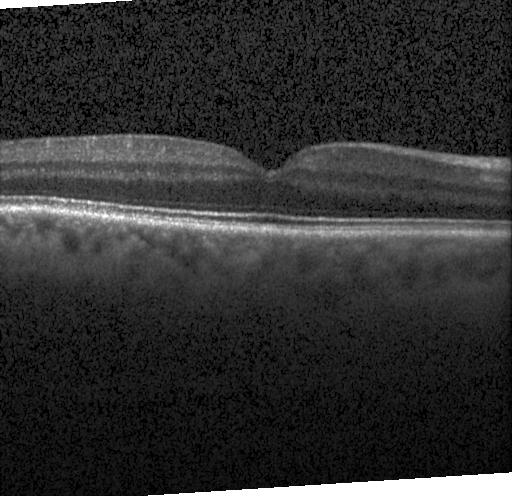

OCT finding: no choroidal neovascularization, no diabetic macular edema, and no drusen.